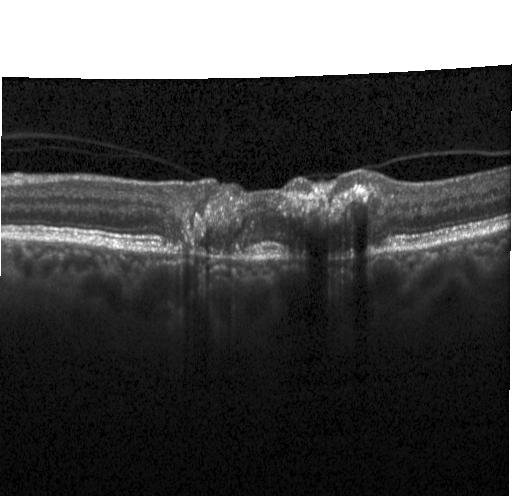 OCT finding: a choroidal neovascular membrane.